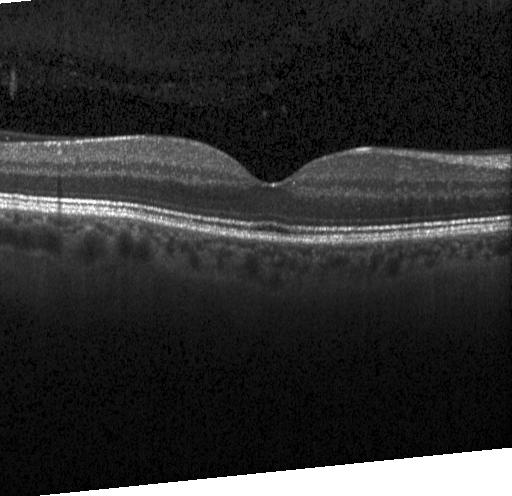 OCT line scan.
Macular OCT: no choroidal neovascularization, diabetic macular edema, or drusen.